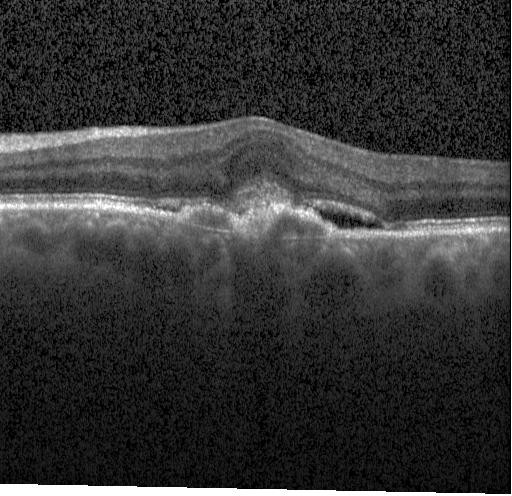

Retinal OCT cross-section · macular scan · spectral-domain OCT · Heidelberg Spectralis.
Diagnosis: choroidal neovascularization.